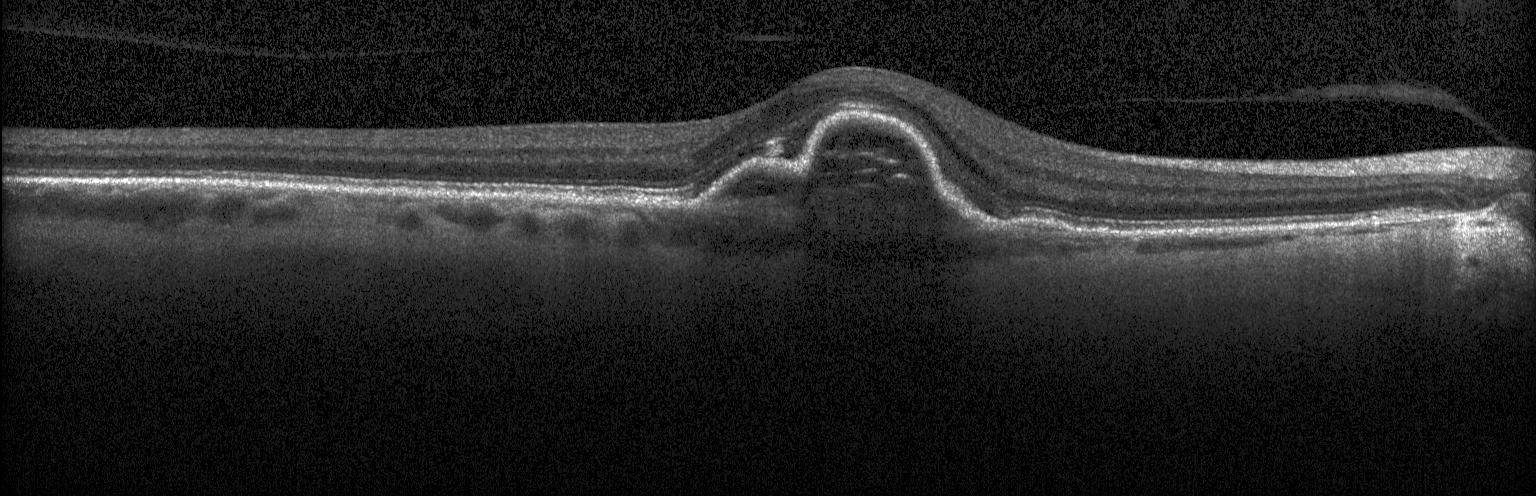 OCT B-scan
The scan shows CNV.